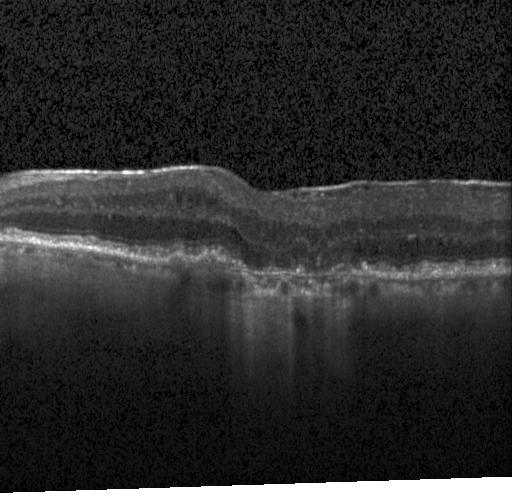 Acquired on a Heidelberg Spectralis. Retinal OCT cross-section. Finding: a choroidal neovascular membrane.